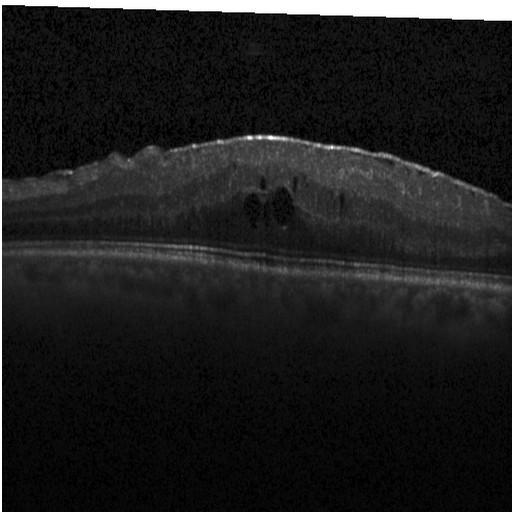
Spectral-domain OCT. Instrument: Heidelberg Spectralis. OCT line scan. Fovea-centered.
Assessment: DME.